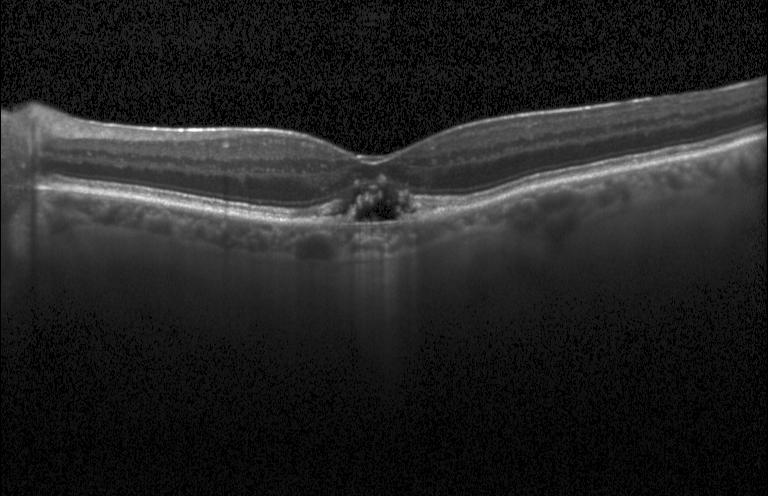

OCT B-scan. Impression: CNV.